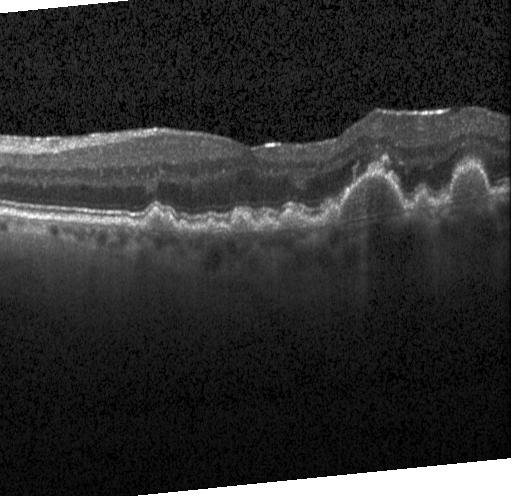

Optical coherence tomography B-scan; SD-OCT; instrument: Heidelberg Spectralis.
Finding: sub-RPE drusenoid deposits.